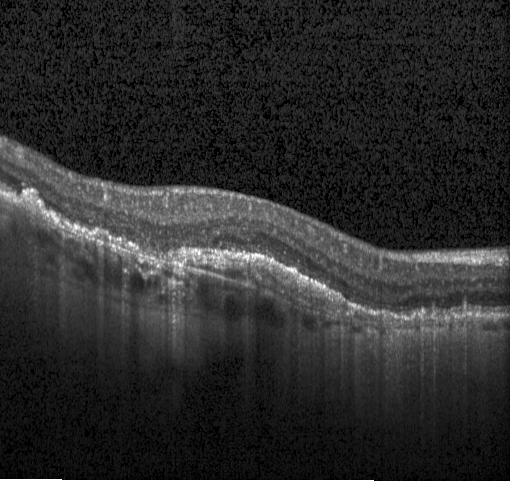

Fovea-centered · spectral-domain OCT · optical coherence tomography B-scan · Heidelberg Spectralis OCT system — Impression: a choroidal neovascular membrane.